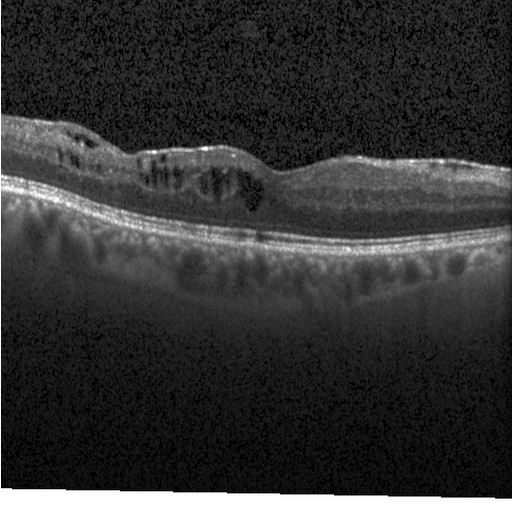 Instrument: Heidelberg Spectralis · OCT line scan · macular scan · spectral-domain optical coherence tomography
Assessment: DME.